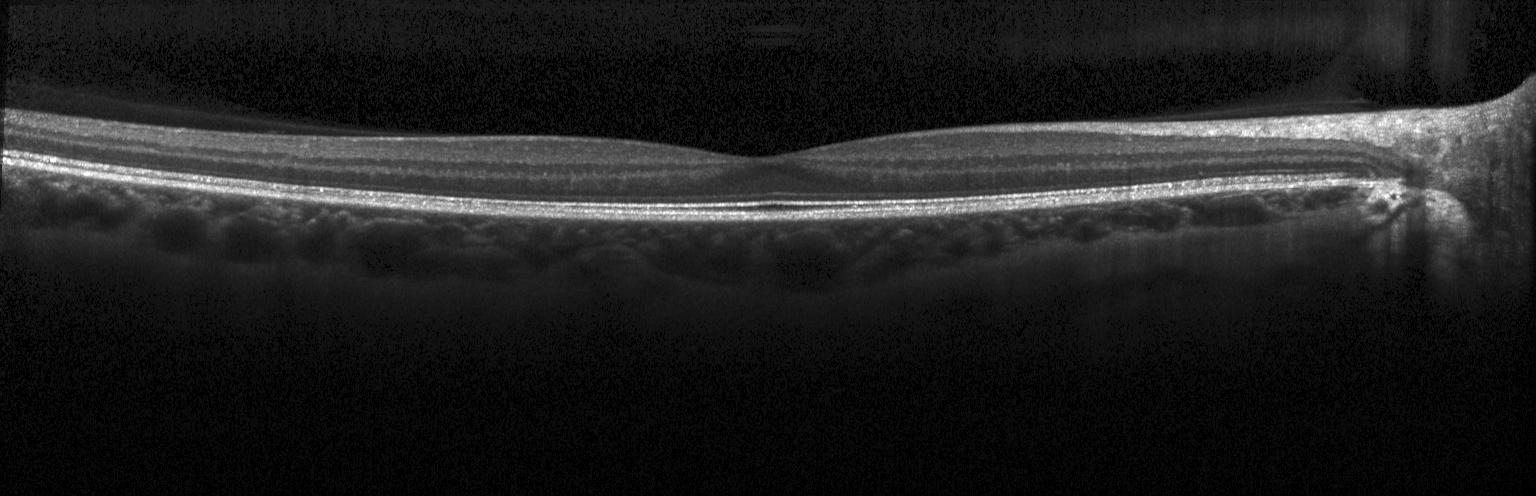
Heidelberg Spectralis OCT system. Retinal OCT cross-section.
Impression: no CNV, DME, or drusen.